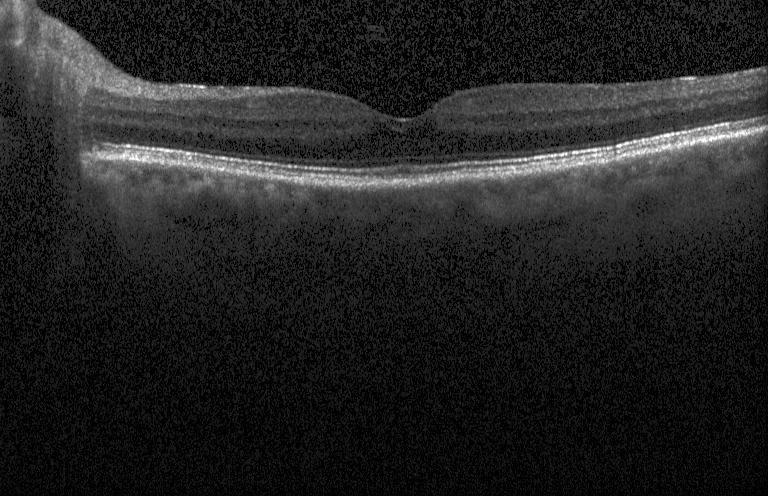
OCT B-scan; Heidelberg Spectralis OCT system; centered on the fovea
Diagnosis: no choroidal neovascularization, diabetic macular edema, or drusen.